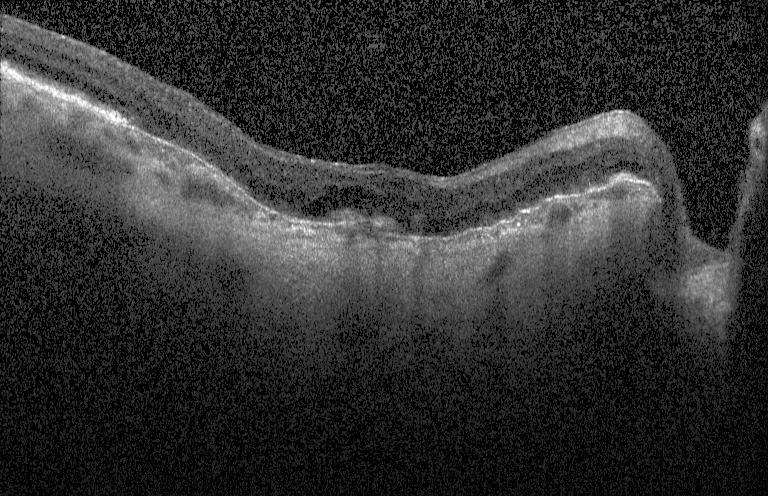
Assessment: CNV.